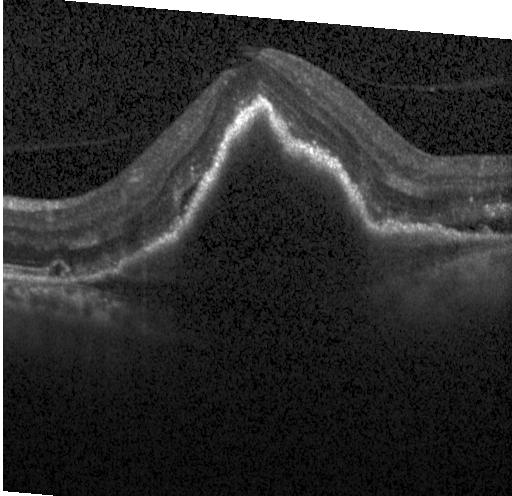
The scan shows a choroidal neovascular membrane.